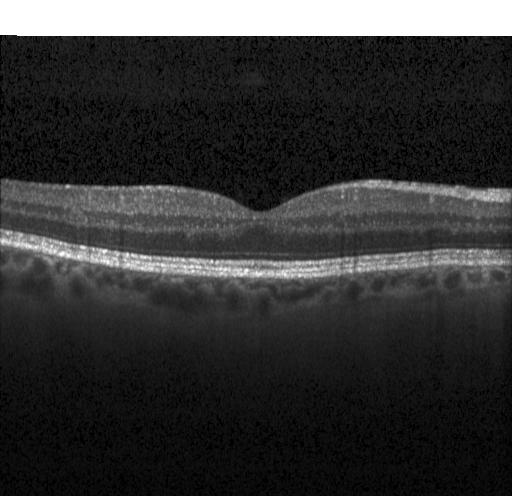

Macular OCT: no evidence of choroidal neovascularization, diabetic macular edema, or drusen.